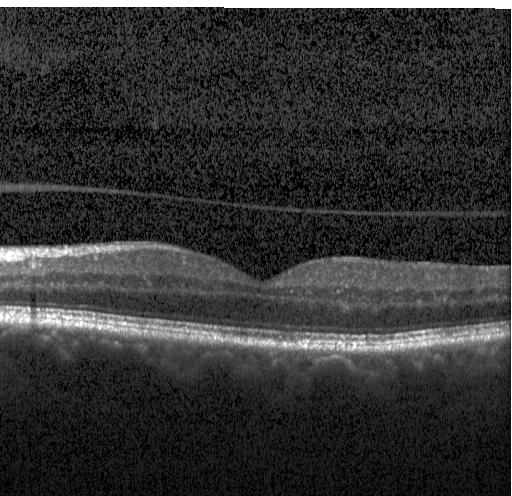 OCT scan showing no evidence of choroidal neovascularization, diabetic macular edema, or drusen.